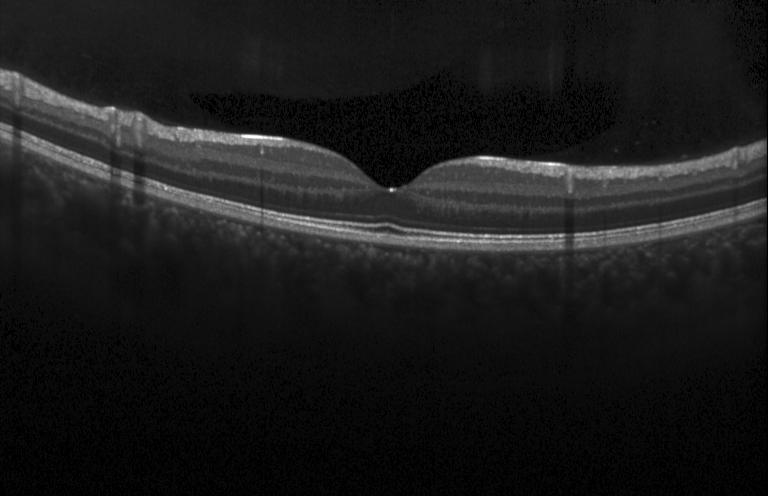
Impression: neither choroidal neovascularization, diabetic macular edema, nor drusen.